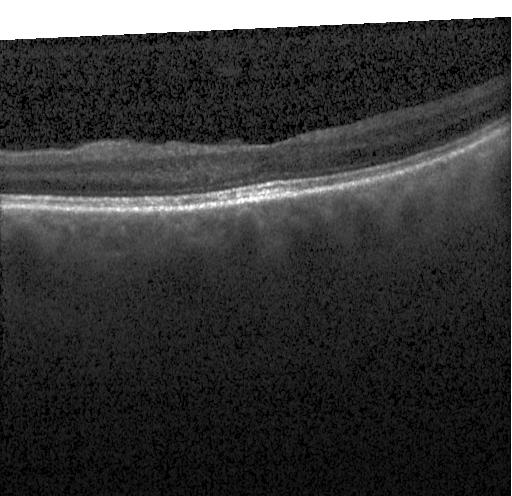

Macular OCT demonstrating no choroidal neovascularization, diabetic macular edema, or drusen.